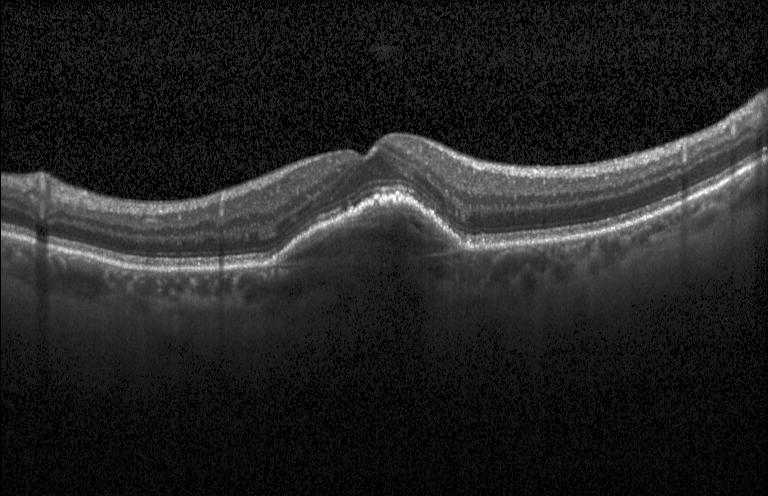

Retinal OCT cross-section. Horizontal scan through the fovea.
Impression: a choroidal neovascular membrane.